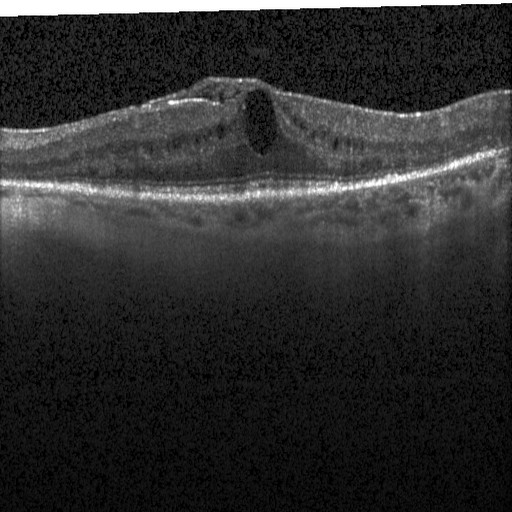
Impression: DME.